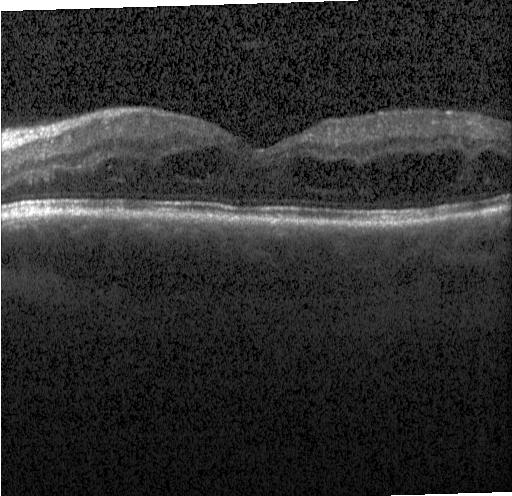 Heidelberg Spectralis, spectral-domain OCT, retinal OCT B-scan
Finding: diabetic macular edema (DME).